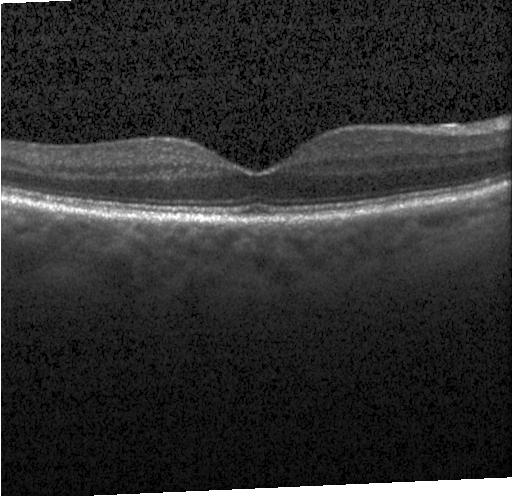
SD-OCT · optical coherence tomography B-scan — Finding: no CNV, no DME, and no drusen.